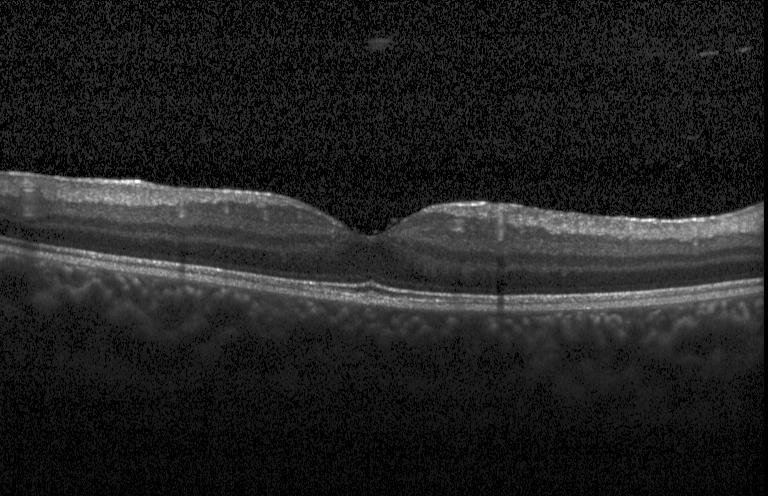

Spectral-domain OCT; acquired on a Heidelberg Spectralis; fovea-centered; OCT line scan.
OCT finding: no CNV, no DME, and no drusen.